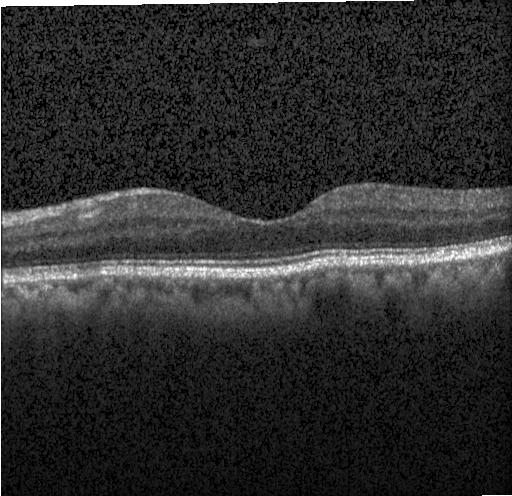 OCT B-scan, centered on the fovea. Dx: no evidence of choroidal neovascularization, diabetic macular edema, or drusen.